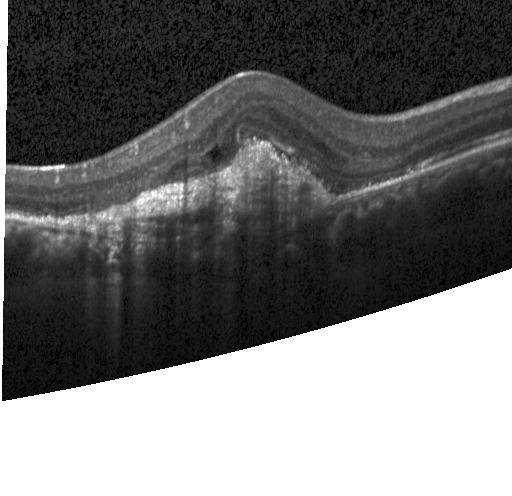 Retinal OCT cross-section; SD-OCT. Diagnosis: a choroidal neovascular membrane.